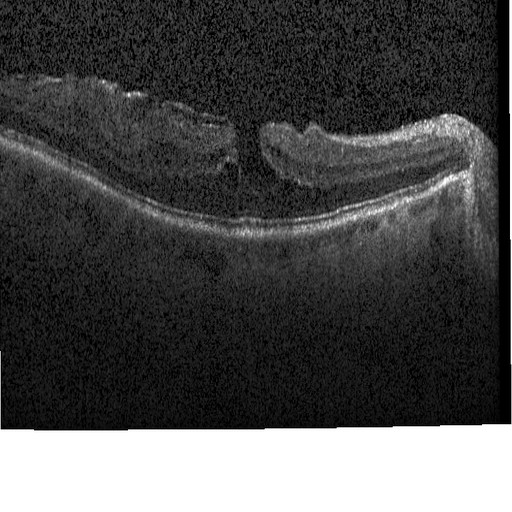
Retinal OCT cross-section — Diabetic macular edema.